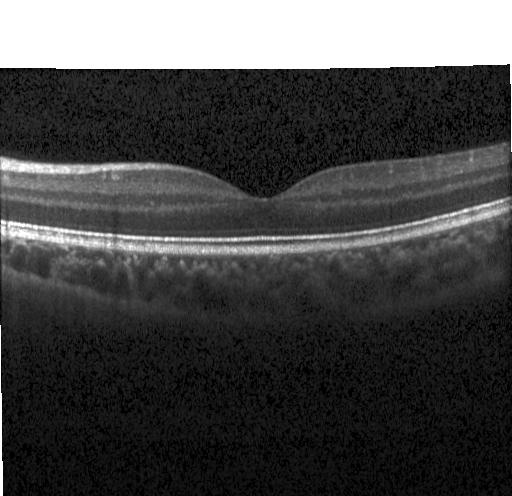 Retinal OCT B-scan, spectral-domain optical coherence tomography, centered on the fovea
The scan shows no choroidal neovascularization, no diabetic macular edema, and no drusen.